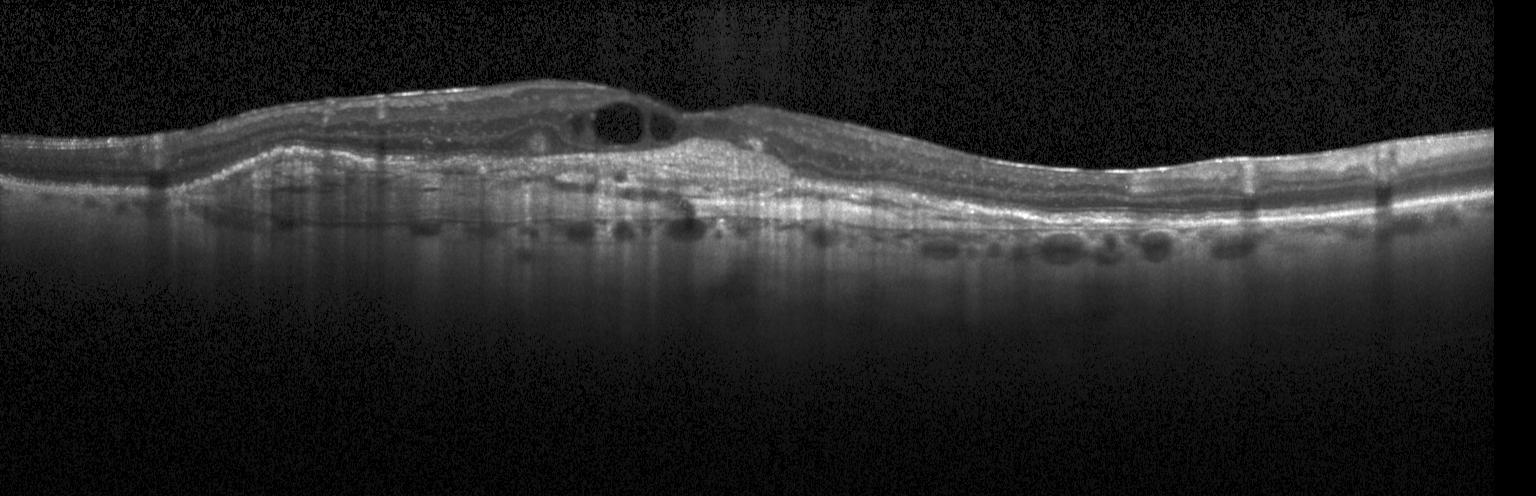 Impression: a choroidal neovascular membrane.